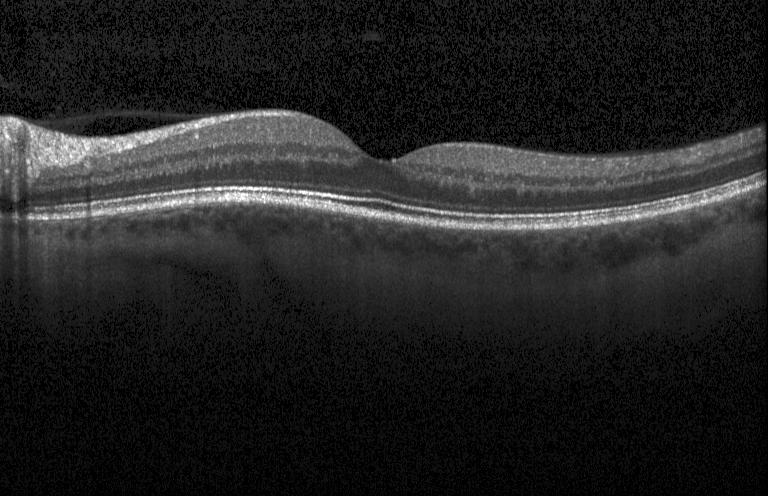 Impression: no evidence of choroidal neovascularization, diabetic macular edema, or drusen.